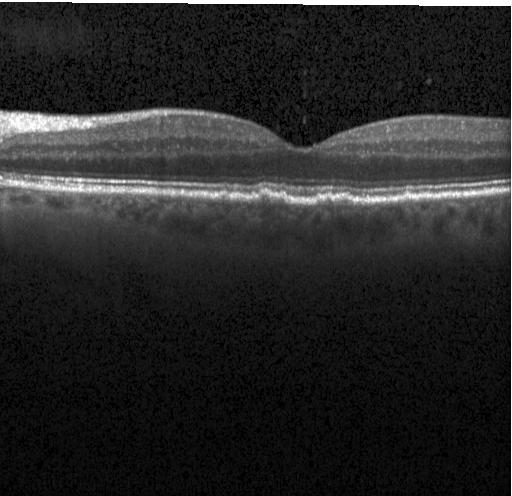 OCT B-scan.
Finding: drusen.